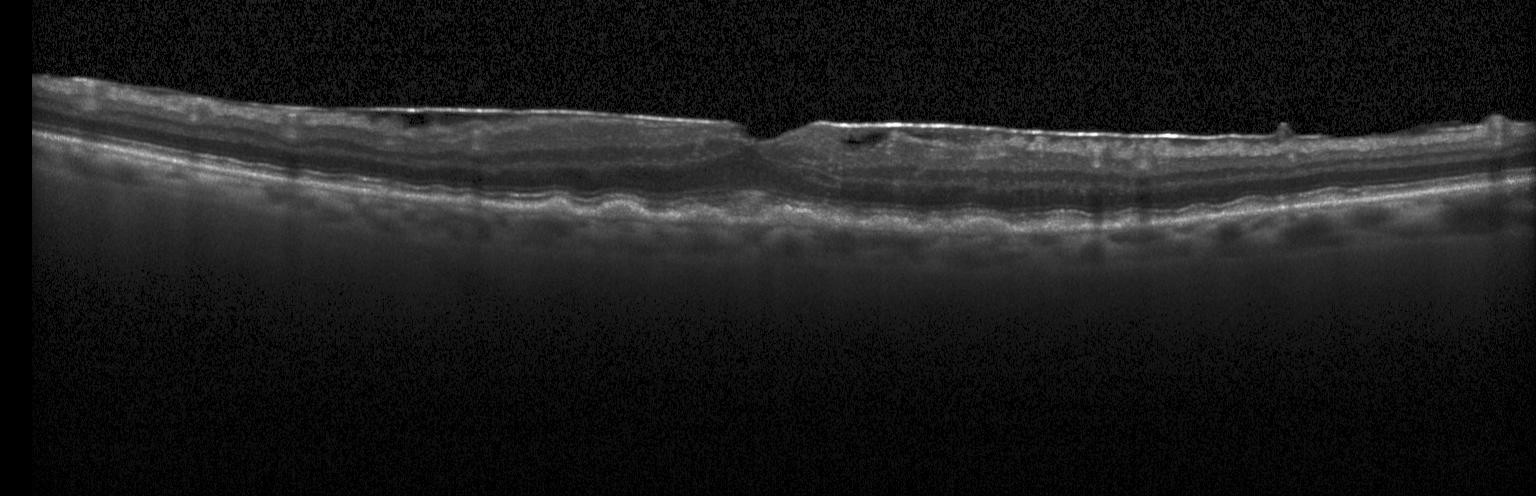 Spectral-domain OCT; retinal OCT B-scan
Dx: sub-RPE drusenoid deposits.